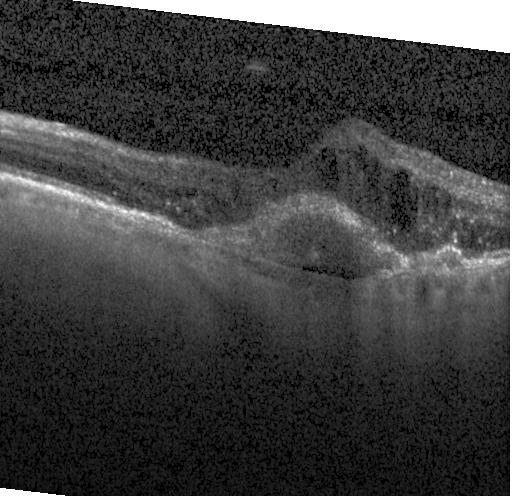

OCT B-scan
OCT finding: a choroidal neovascular membrane.